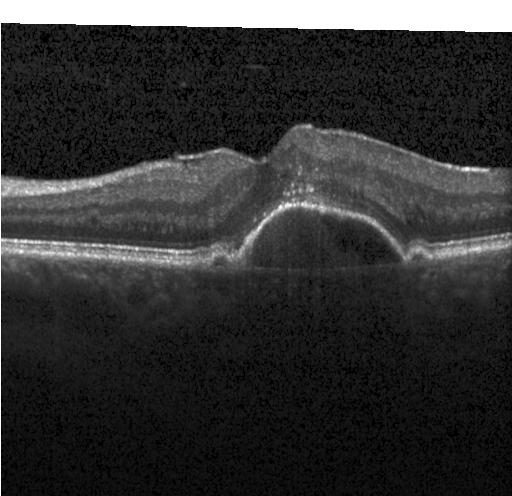
Assessment: a choroidal neovascular membrane.